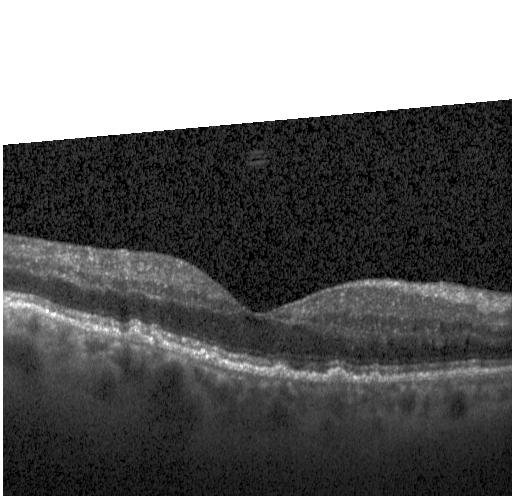 Macular OCT demonstrating multiple drusen.